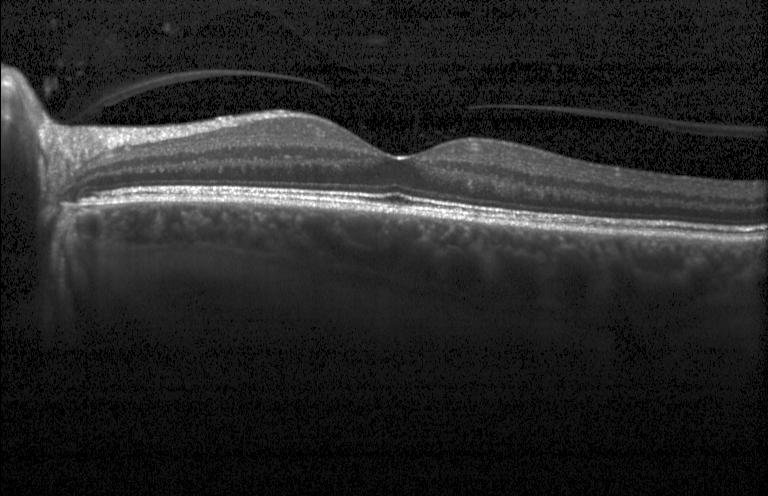 Macular OCT demonstrating no CNV, no DME, and no drusen.